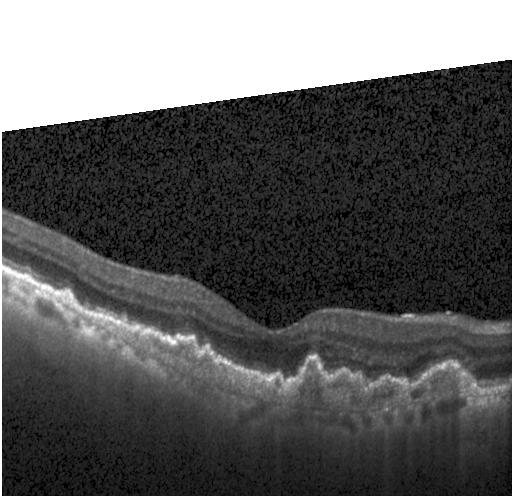 Horizontal scan through the fovea · spectral-domain optical coherence tomography · OCT line scan. Finding: choroidal neovascularization.